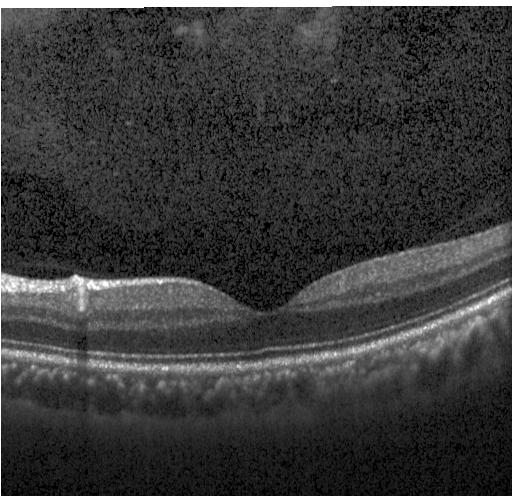
Optical coherence tomography scan; Heidelberg Spectralis OCT system; spectral-domain optical coherence tomography; horizontal scan through the fovea
Finding: no evidence of choroidal neovascularization, diabetic macular edema, or drusen.